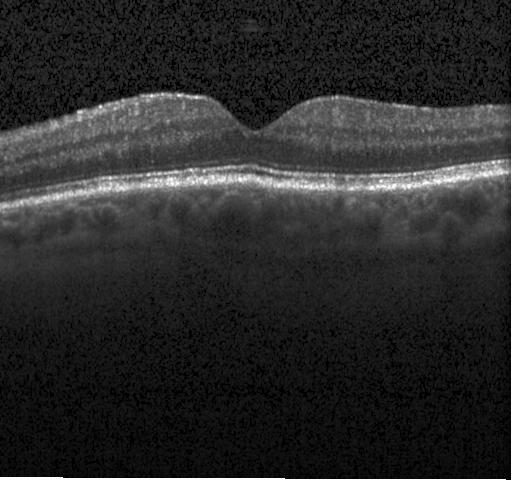
Macular OCT demonstrating no CNV, DME, or drusen.